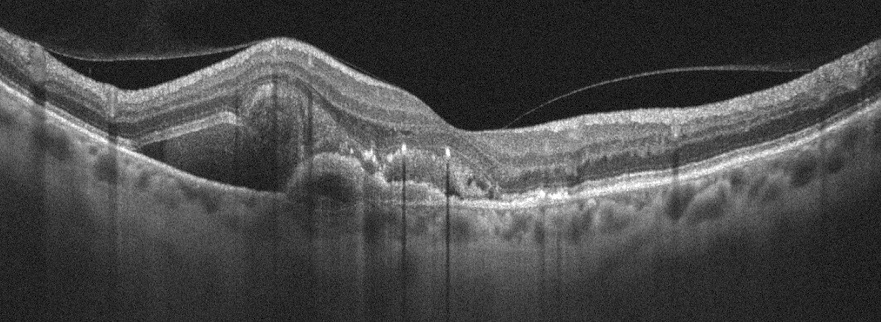 Optical coherence tomography scan
Assessment: AMD.